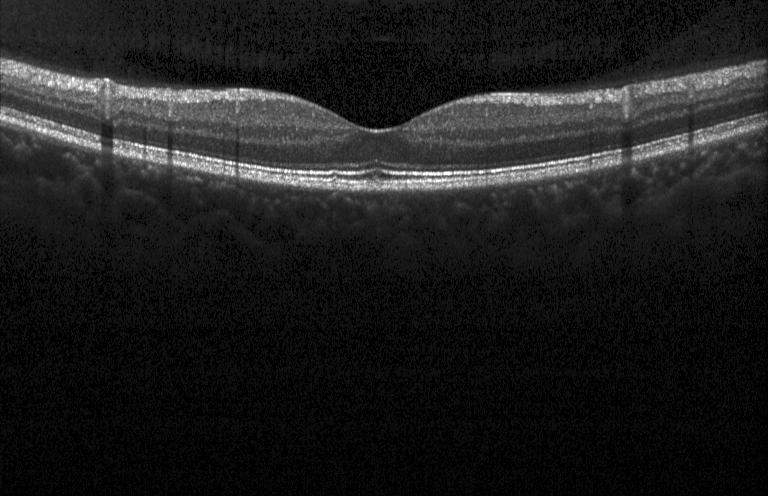

Optical coherence tomography B-scan. Impression: no choroidal neovascularization, no diabetic macular edema, and no drusen.